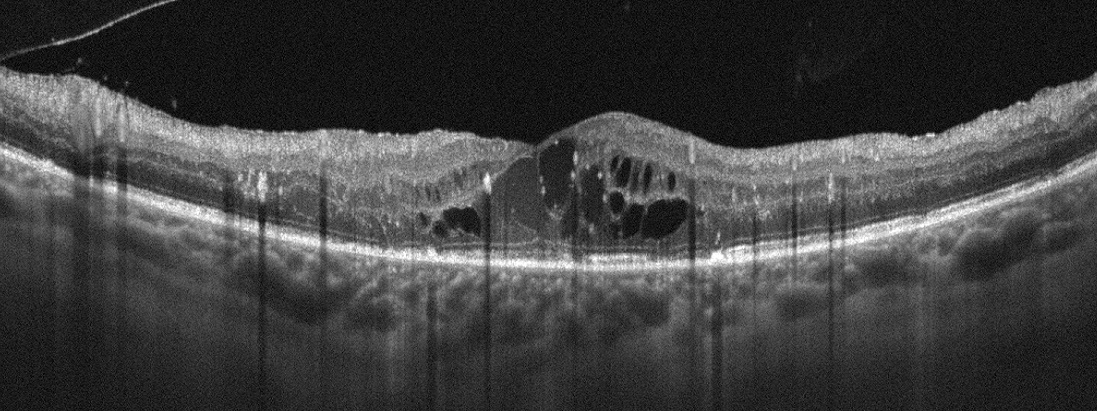

Optical coherence tomography B-scan
Macular OCT: diabetic macular edema.